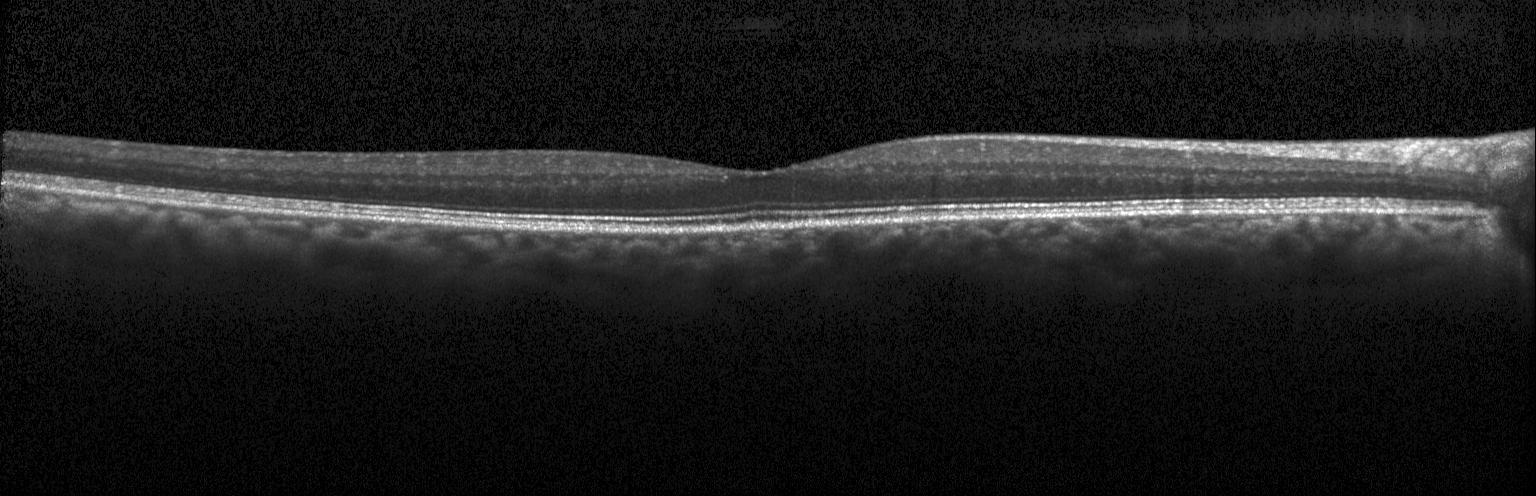

OCT scan showing neither choroidal neovascularization, diabetic macular edema, nor drusen.